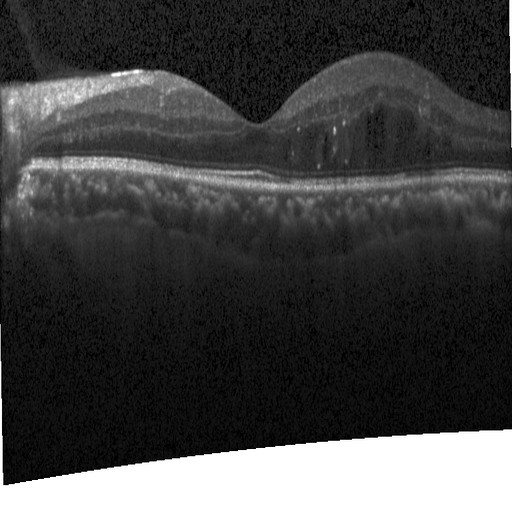
Through the macula. OCT B-scan. Heidelberg Spectralis — Finding: DME.